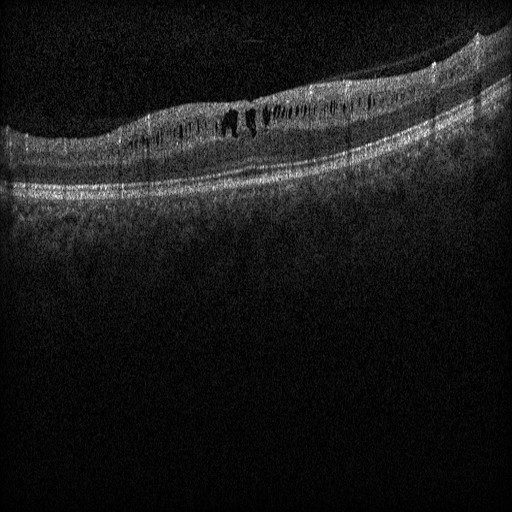
Impression: DME.